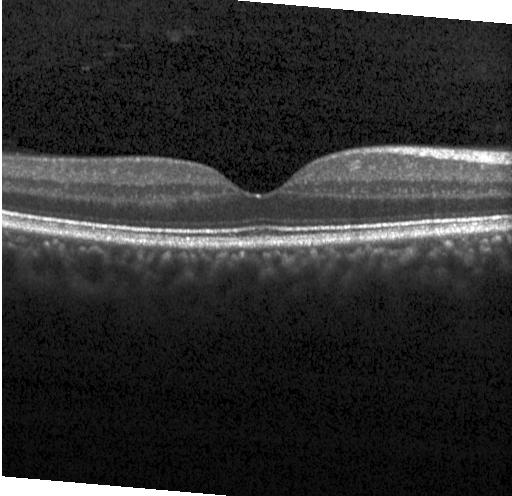 OCT line scan. Impression: neither CNV, DME, nor drusen.